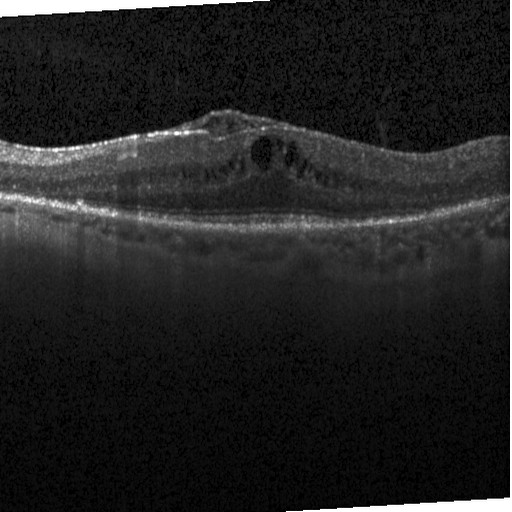 Heidelberg Spectralis · retinal OCT B-scan.
Assessment: diabetic macular edema.